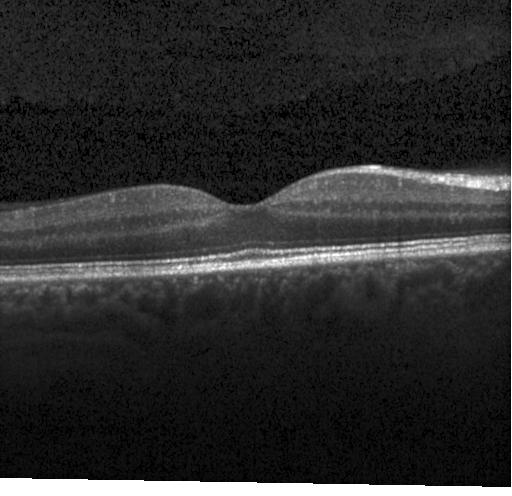 OCT B-scan.
Finding: no choroidal neovascularization, diabetic macular edema, or drusen.